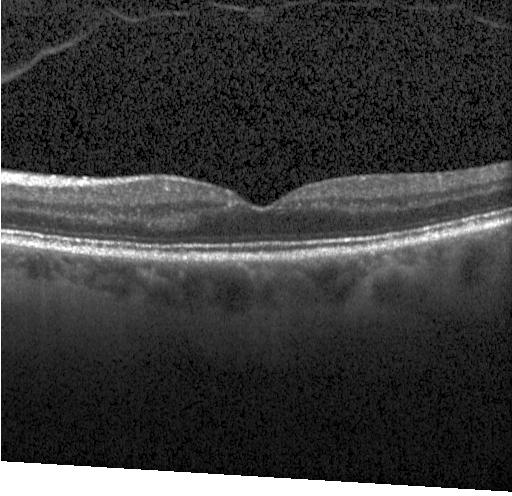 Optical coherence tomography B-scan. Impression: no choroidal neovascularization, diabetic macular edema, or drusen.